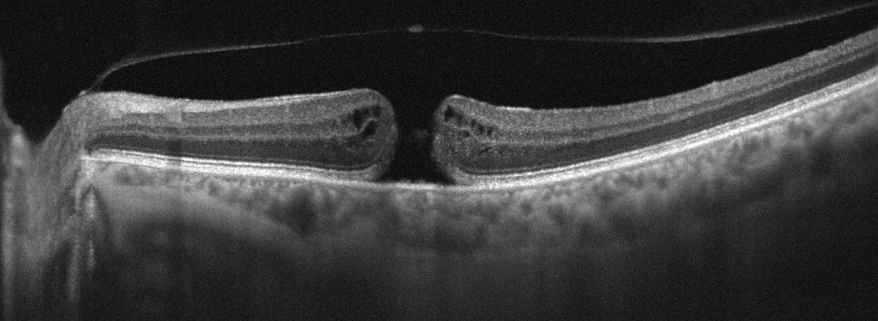

OCT B-scan showing VID.